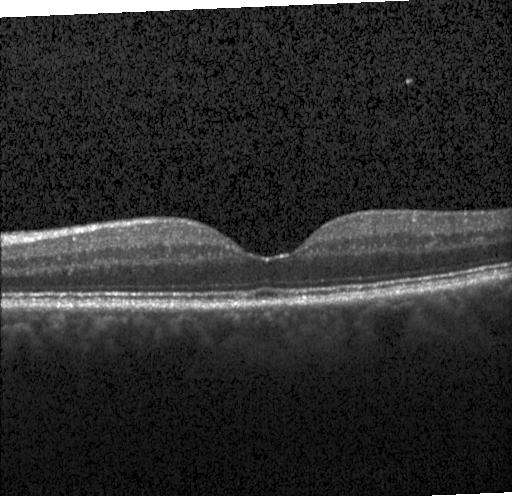
Acquired on a Heidelberg Spectralis, SD-OCT, retinal OCT B-scan, fovea-centered — Dx: neither choroidal neovascularization, diabetic macular edema, nor drusen.